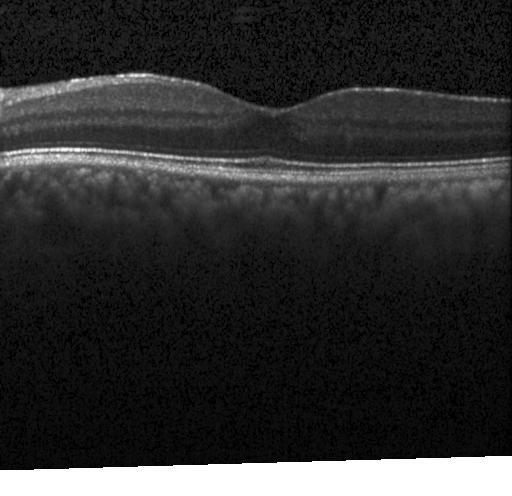
OCT line scan · instrument: Heidelberg Spectralis. This B-scan demonstrates neither CNV, DME, nor drusen.